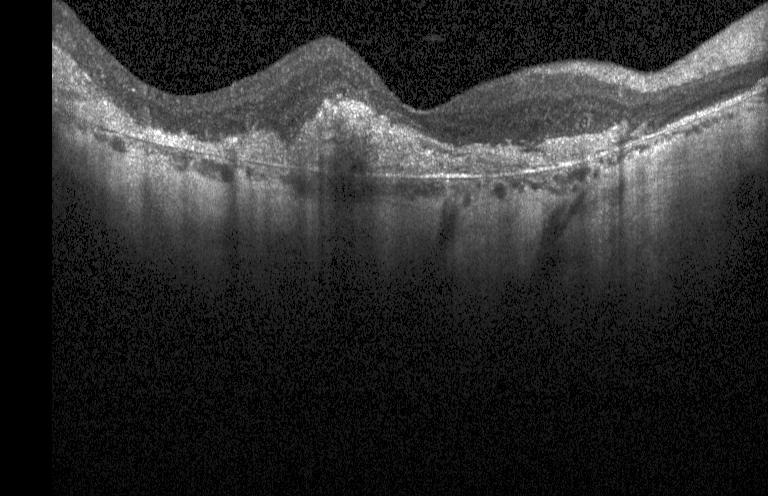
Horizontal scan through the fovea; SD-OCT; retinal OCT cross-section; Heidelberg Spectralis
Dx: choroidal neovascularization (CNV).